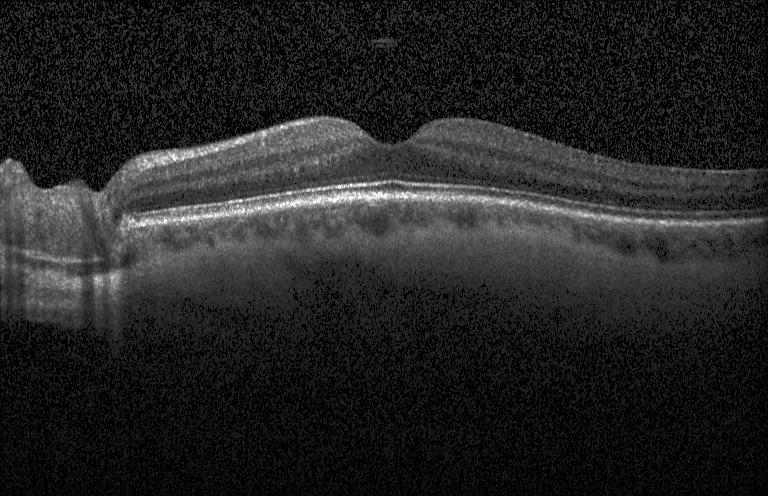 Optical coherence tomography B-scan.
Dx: no evidence of choroidal neovascularization, diabetic macular edema, or drusen.